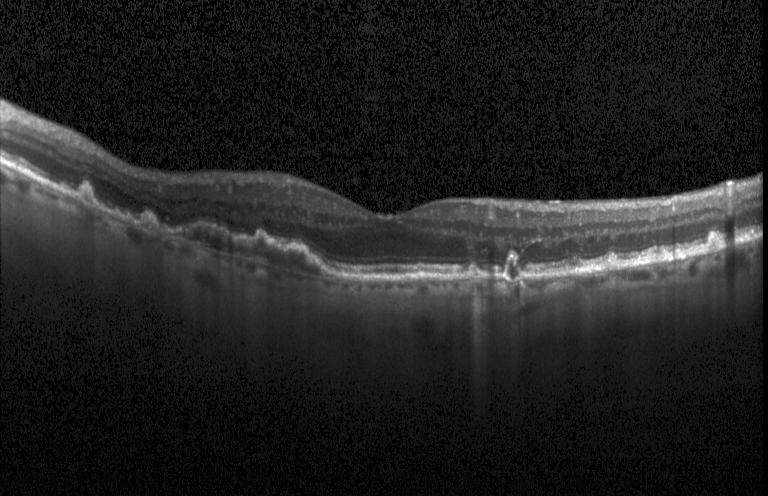

OCT line scan; macular scan
Finding: choroidal neovascularization (CNV).